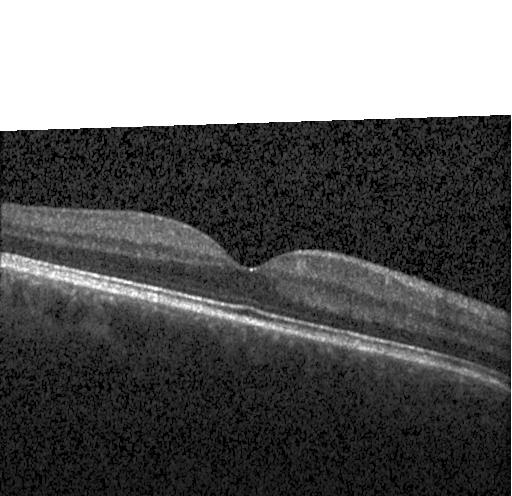 OCT line scan; centered on the fovea.
This B-scan demonstrates no choroidal neovascularization, diabetic macular edema, or drusen.